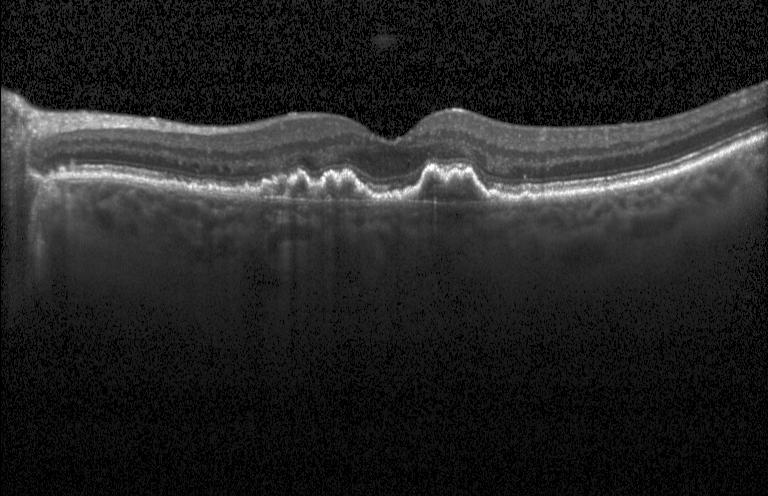

Retinal OCT cross-section. Macular scan. Acquired on a Heidelberg Spectralis
Assessment: a choroidal neovascular membrane.